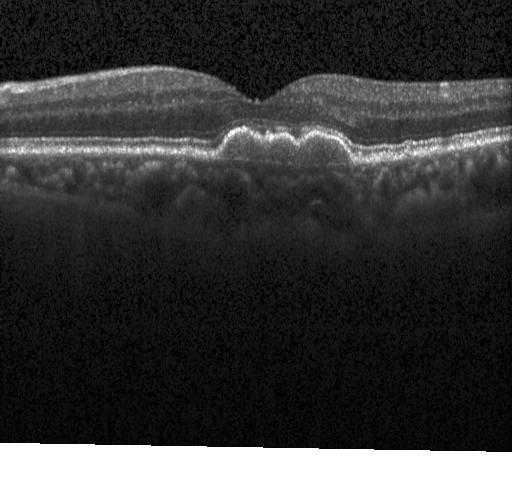 Fovea-centered, optical coherence tomography scan. The scan shows sub-RPE drusenoid deposits.